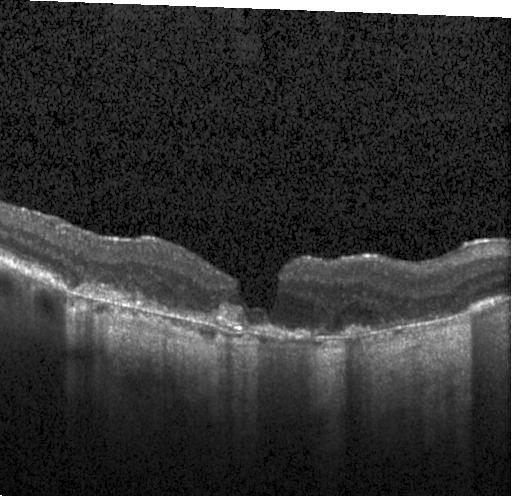

Retinal OCT cross-section.
Diagnosis: a choroidal neovascular membrane.